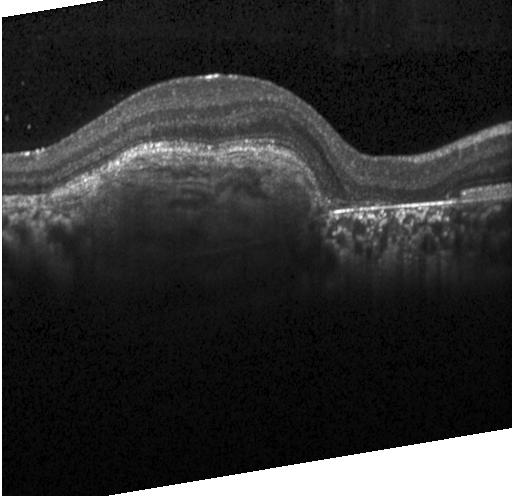 This B-scan demonstrates a choroidal neovascular membrane.